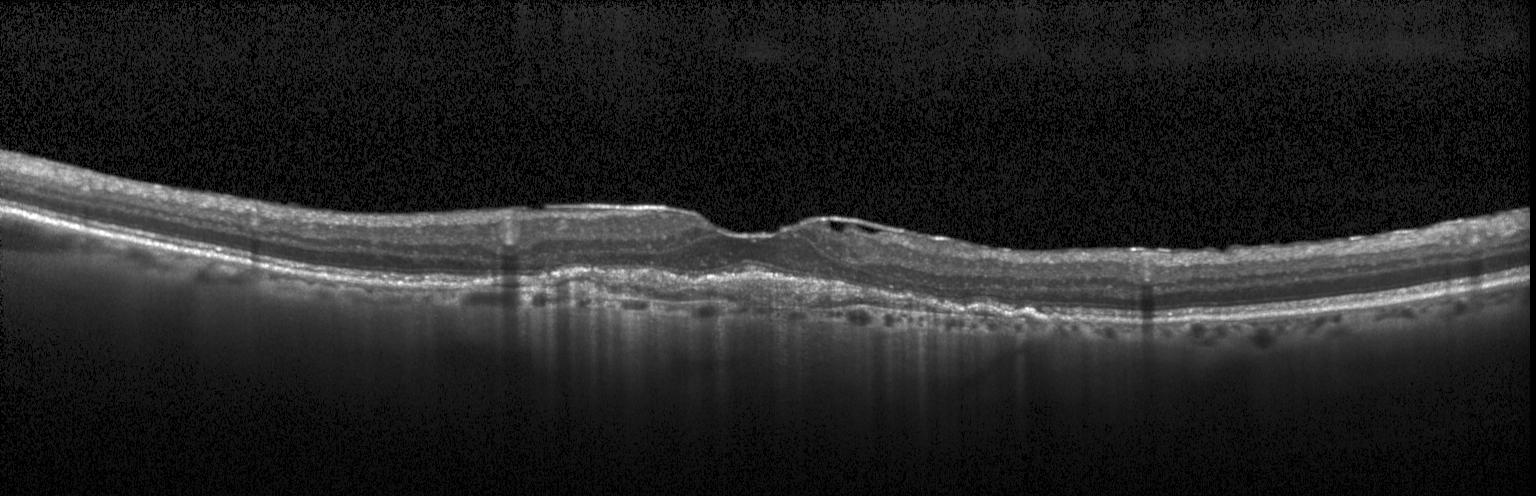 Diagnosis: choroidal neovascularization (CNV).